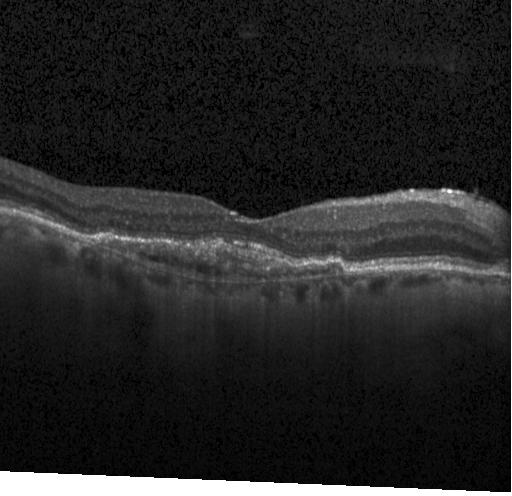 Macular OCT: a choroidal neovascular membrane.